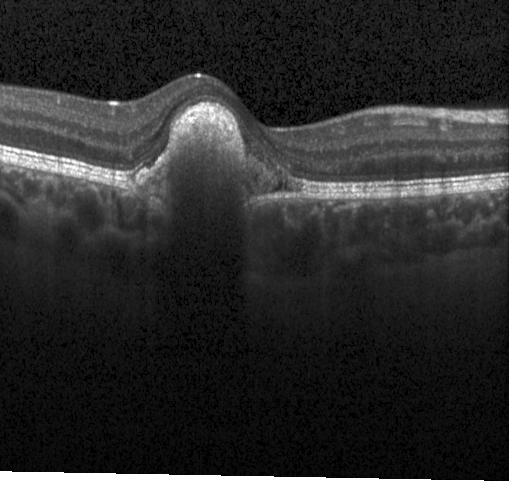 OCT scan showing choroidal neovascularization.